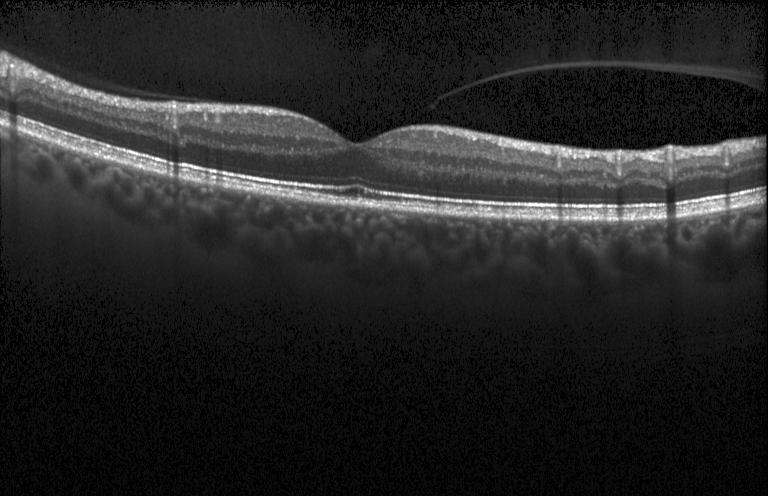 Assessment: no CNV, DME, or drusen.